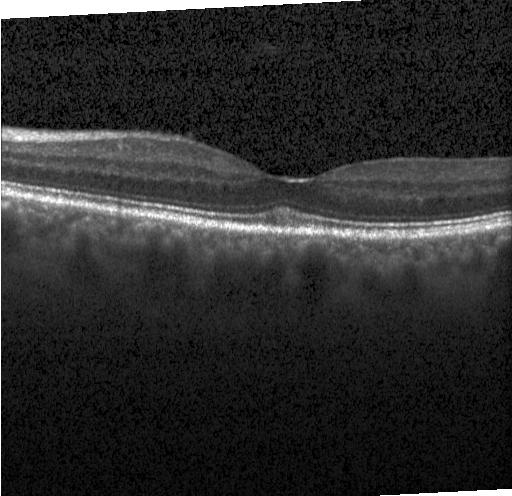 OCT scan showing neither choroidal neovascularization, diabetic macular edema, nor drusen.